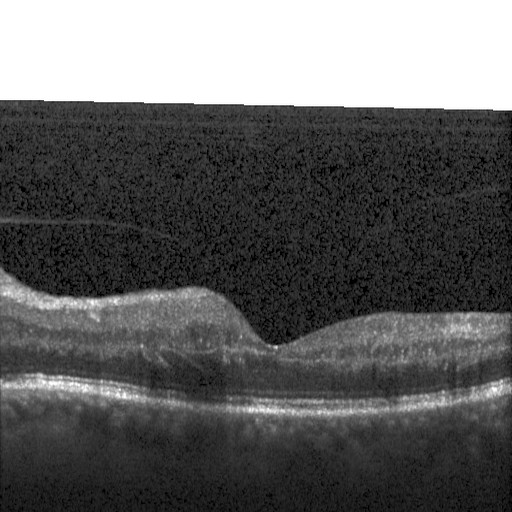

Heidelberg Spectralis; OCT B-scan.
Assessment: diabetic macular edema (DME).